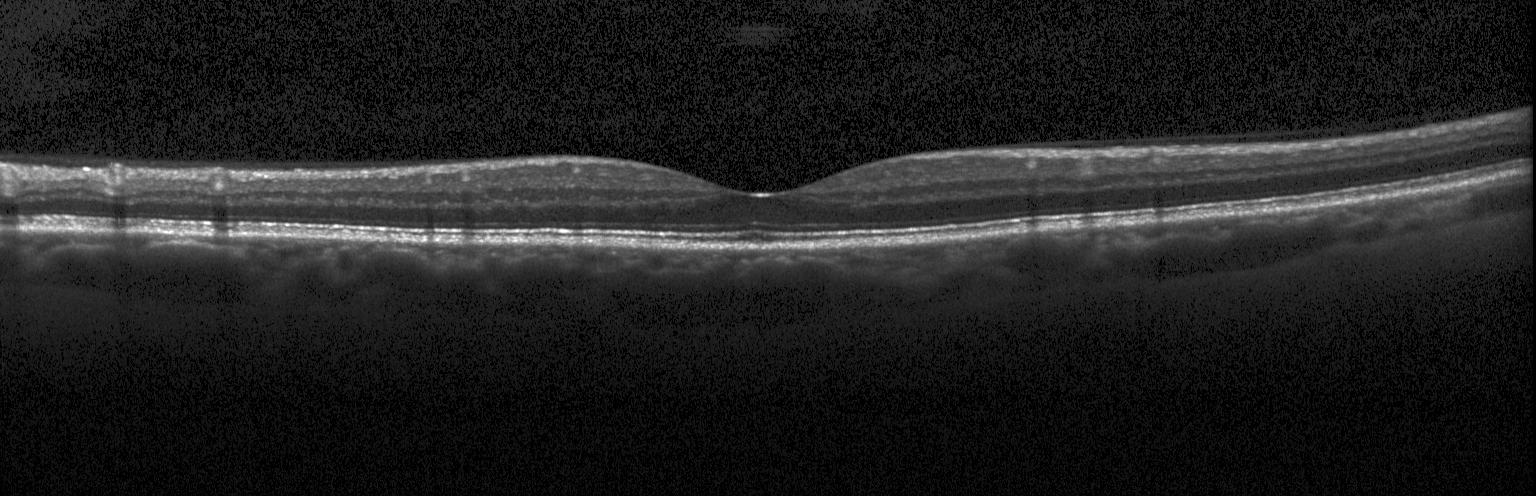
Impression: no evidence of choroidal neovascularization, diabetic macular edema, or drusen.